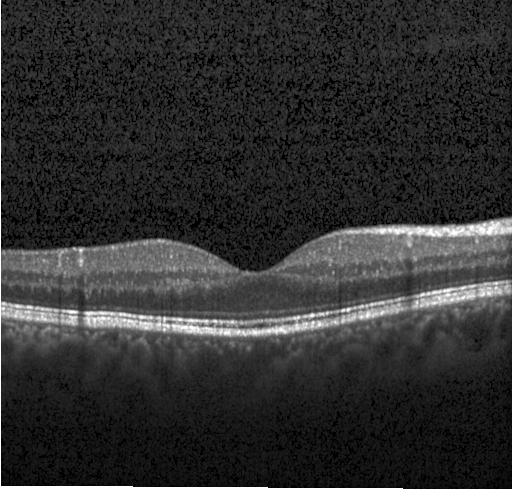
The scan shows neither choroidal neovascularization, diabetic macular edema, nor drusen.